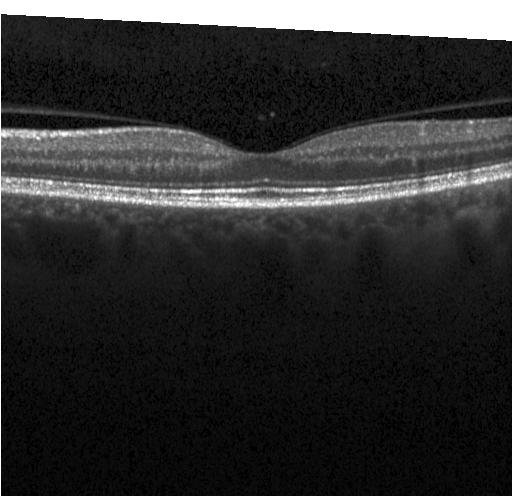

SD-OCT. Acquired on a Heidelberg Spectralis. OCT B-scan.
This B-scan demonstrates no choroidal neovascularization, no diabetic macular edema, and no drusen.